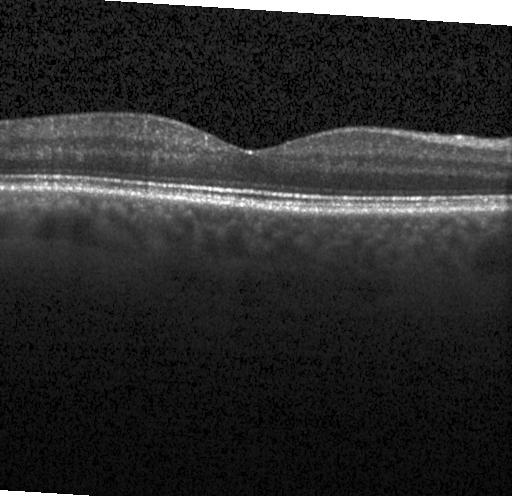
Horizontal scan through the fovea; retinal OCT B-scan; spectral-domain OCT.
Finding: no choroidal neovascularization, diabetic macular edema, or drusen.